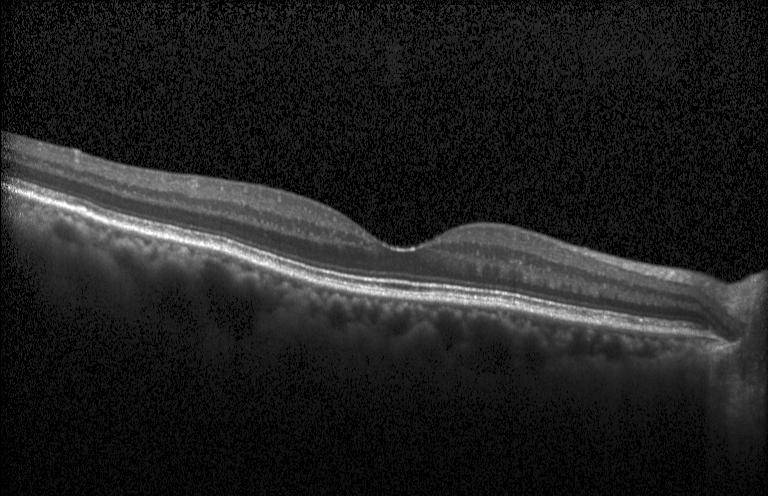
Impression: no choroidal neovascularization, diabetic macular edema, or drusen.